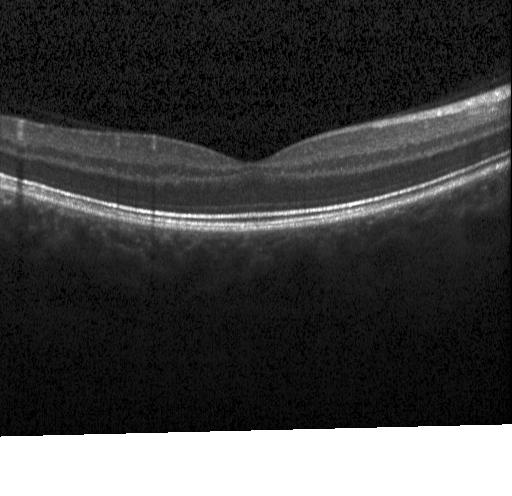
OCT B-scan showing neither choroidal neovascularization, diabetic macular edema, nor drusen.